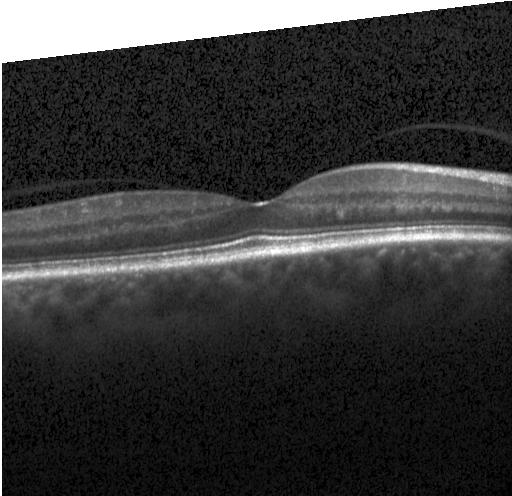 Retinal OCT cross-section showing no choroidal neovascularization, no diabetic macular edema, and no drusen.